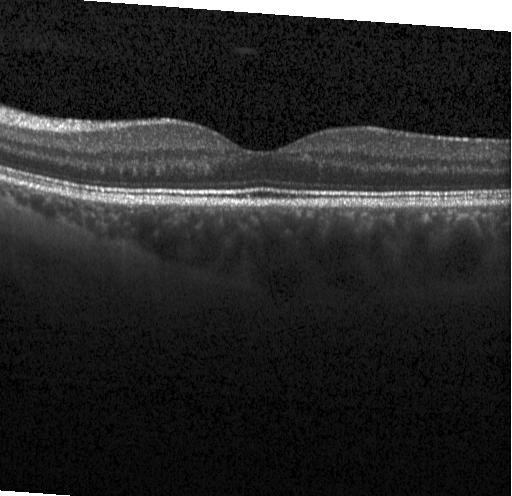
Macular OCT: no evidence of choroidal neovascularization, diabetic macular edema, or drusen.